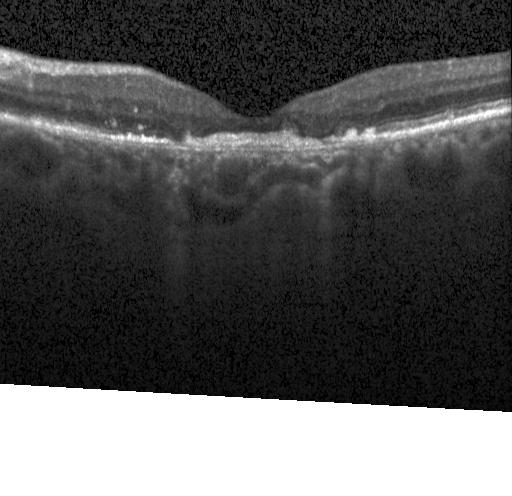 OCT B-scan — Impression: a choroidal neovascular membrane.